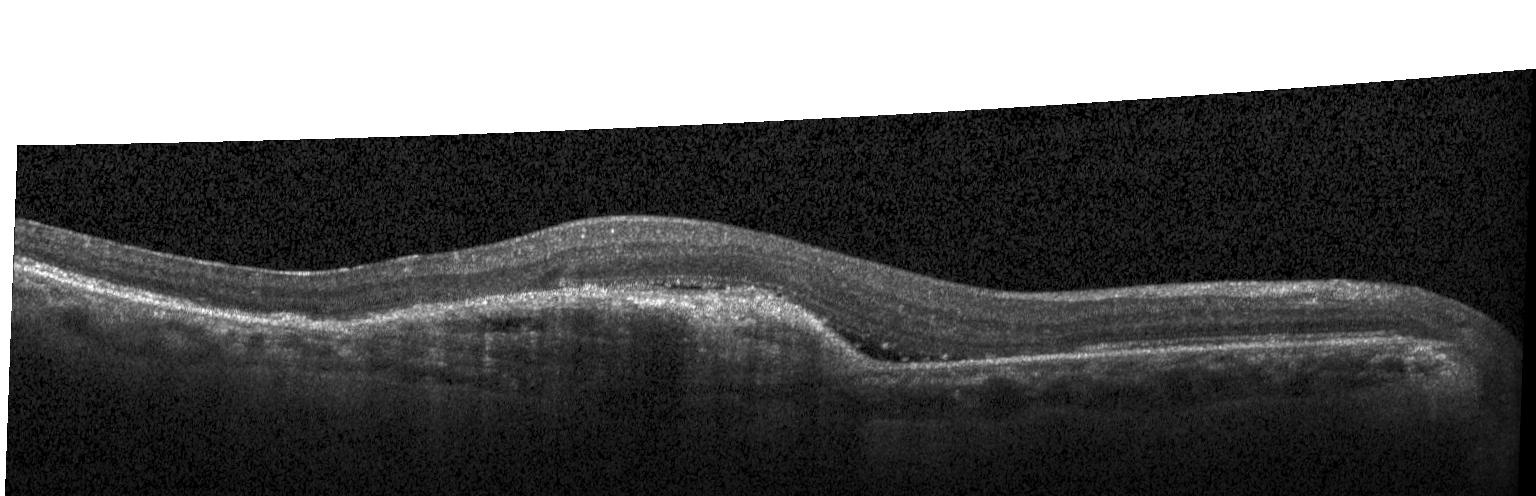

Retinal OCT B-scan. Heidelberg Spectralis OCT system — The scan shows a choroidal neovascular membrane.